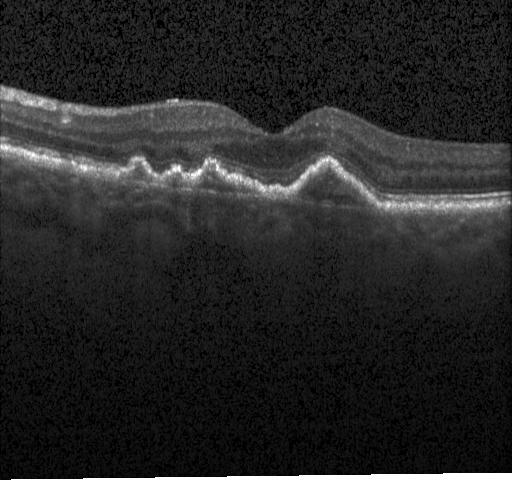 Finding: a choroidal neovascular membrane.